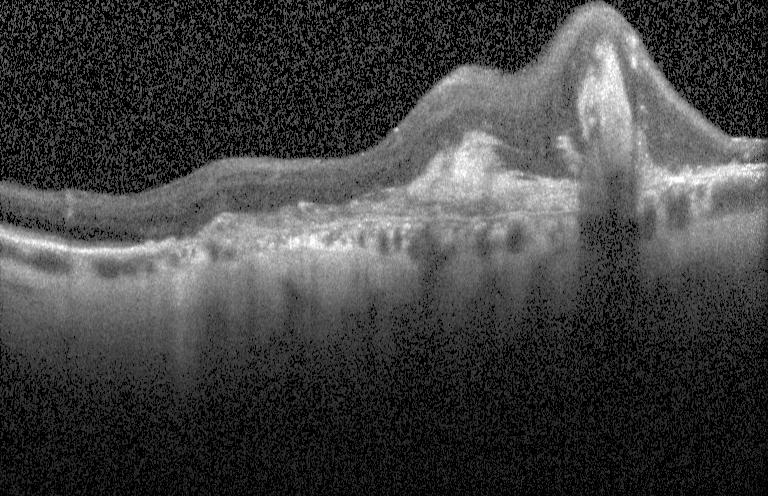 Retinal OCT B-scan — Impression: choroidal neovascularization.